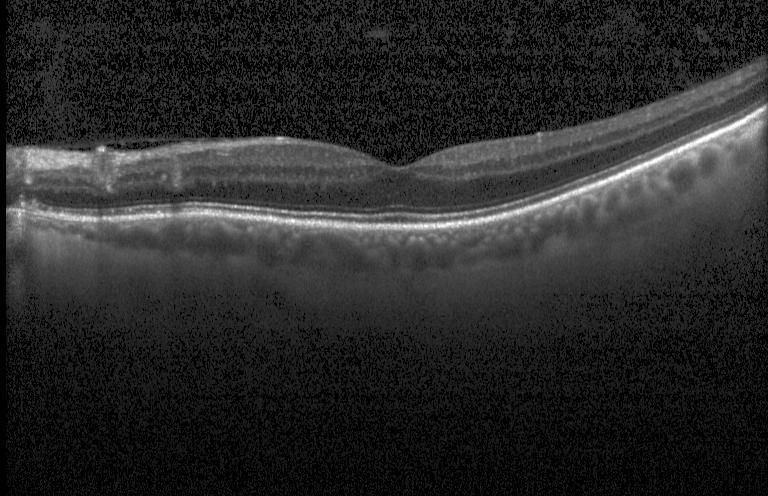 OCT finding: no evidence of CNV, DME, or drusen.